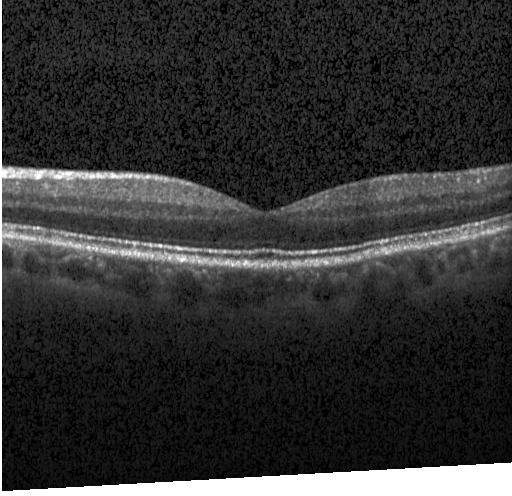

Diagnosis: no evidence of choroidal neovascularization, diabetic macular edema, or drusen.